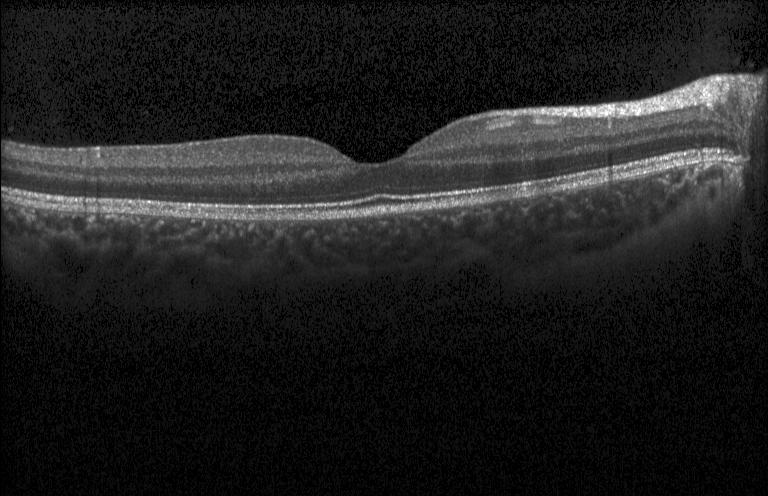
Heidelberg Spectralis OCT system, spectral-domain optical coherence tomography, through the macula, optical coherence tomography scan — Macular OCT: no evidence of choroidal neovascularization, diabetic macular edema, or drusen.